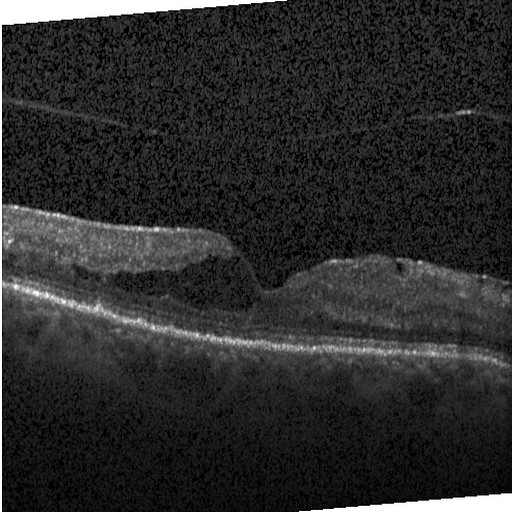
Impression: diabetic macular edema (DME).